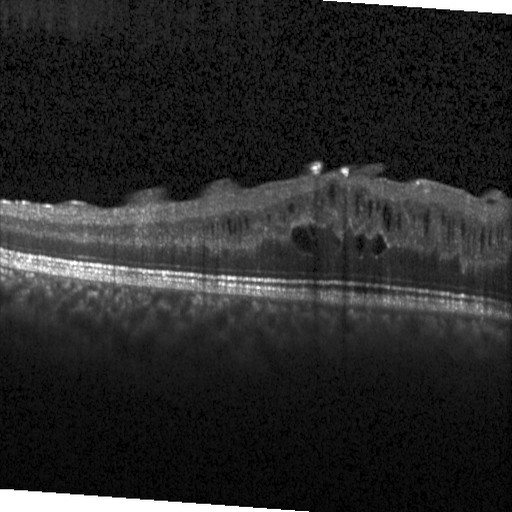
Spectral-domain optical coherence tomography; macular scan; optical coherence tomography B-scan. This B-scan demonstrates diabetic macular edema.